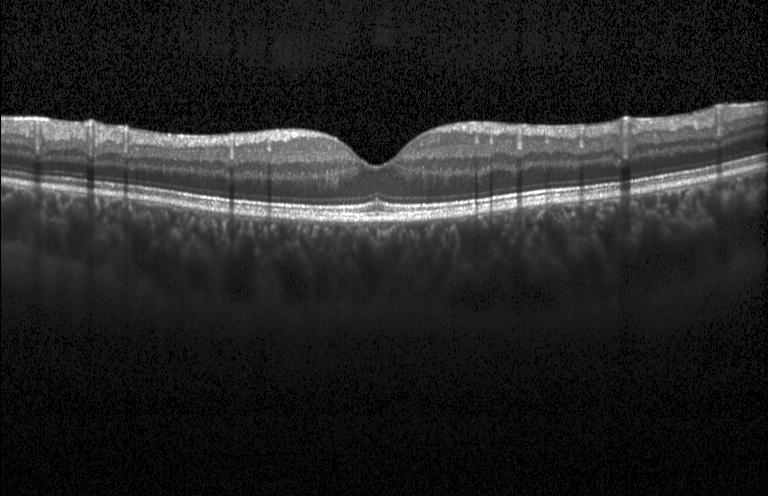

Through the macula · OCT line scan · spectral-domain optical coherence tomography · acquired on a Heidelberg Spectralis. Impression: no choroidal neovascularization, diabetic macular edema, or drusen.